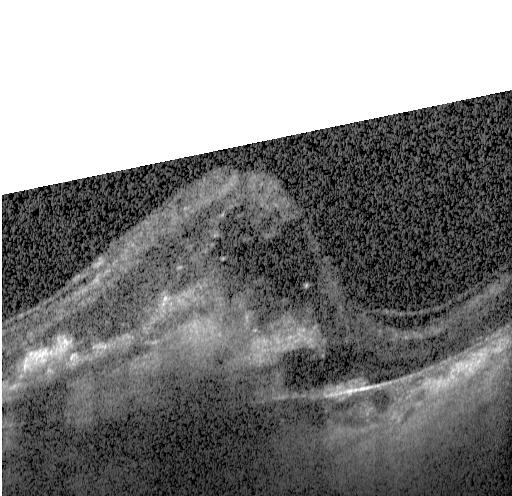

Retinal OCT cross-section, horizontal scan through the fovea. OCT finding: a choroidal neovascular membrane.